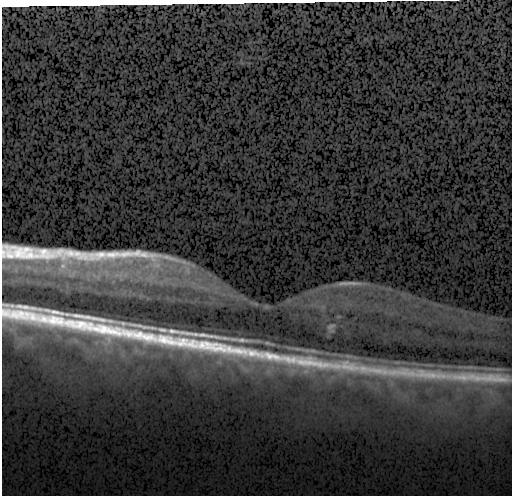
Finding: no evidence of choroidal neovascularization, diabetic macular edema, or drusen.